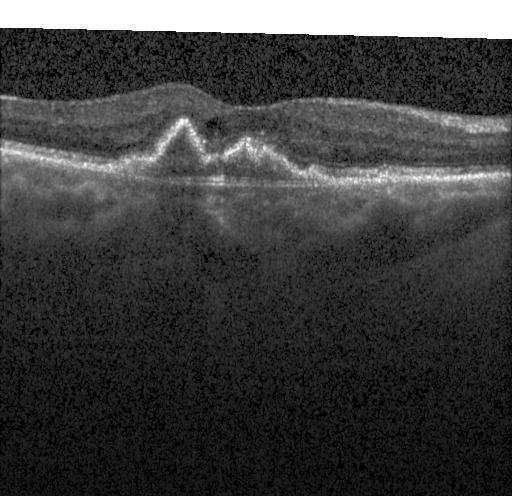

OCT line scan.
Assessment: a choroidal neovascular membrane.